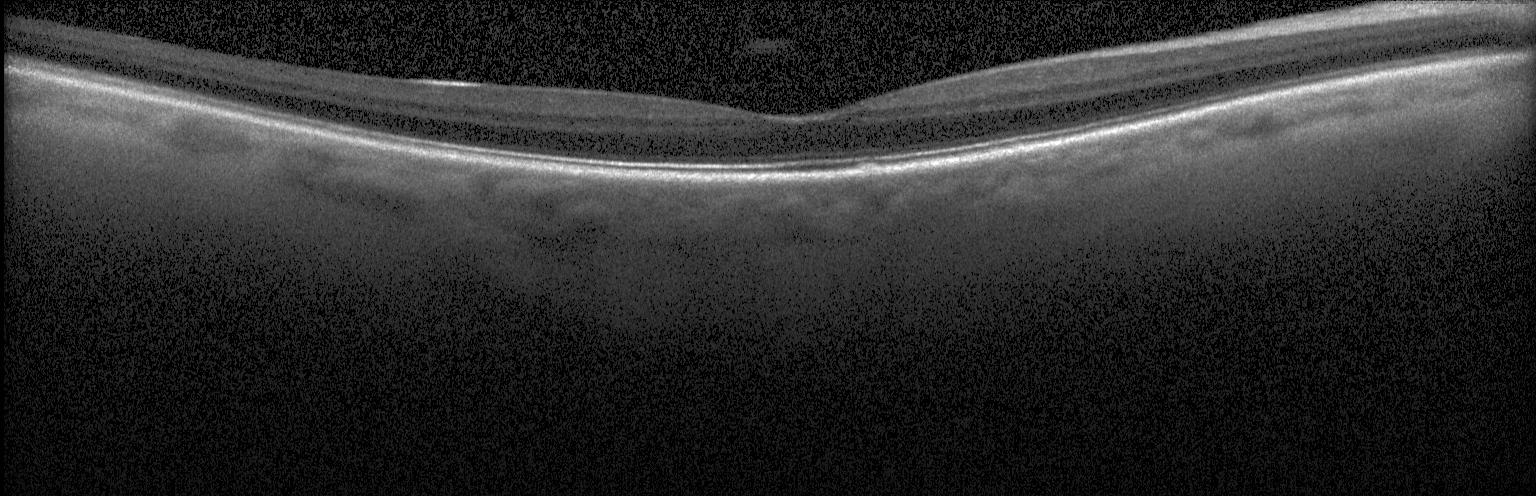
SD-OCT; optical coherence tomography B-scan; through the macula; Heidelberg Spectralis OCT system — The scan shows neither CNV, DME, nor drusen.